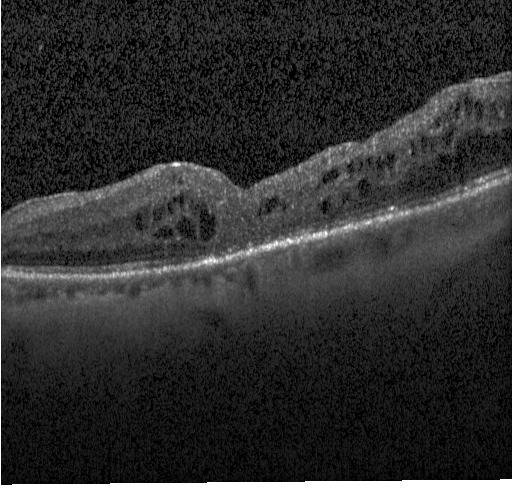

OCT B-scan · Heidelberg Spectralis OCT system · fovea-centered · spectral-domain OCT.
Impression: diabetic macular edema (DME).